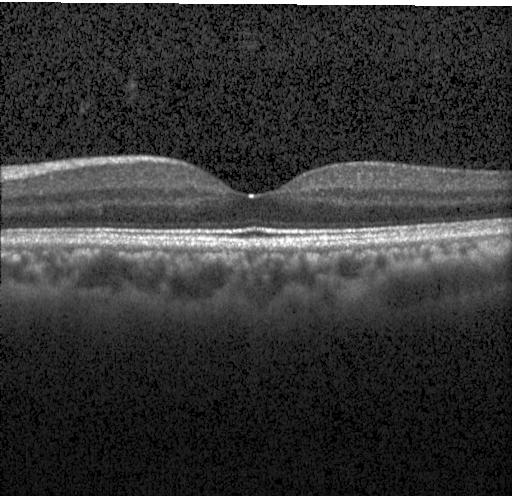 Retinal OCT B-scan.
Finding: neither CNV, DME, nor drusen.